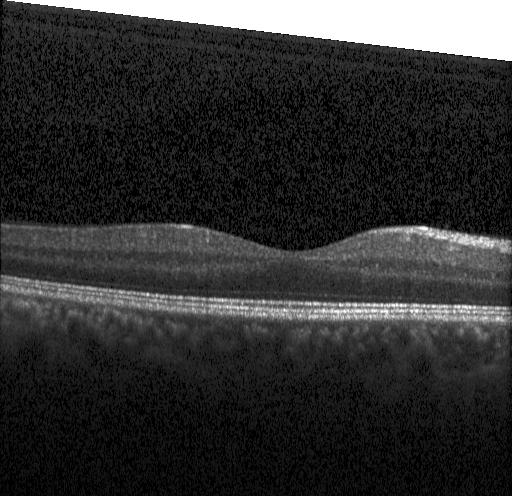

Centered on the fovea; instrument: Heidelberg Spectralis; OCT line scan; spectral-domain OCT
Assessment: no choroidal neovascularization, no diabetic macular edema, and no drusen.